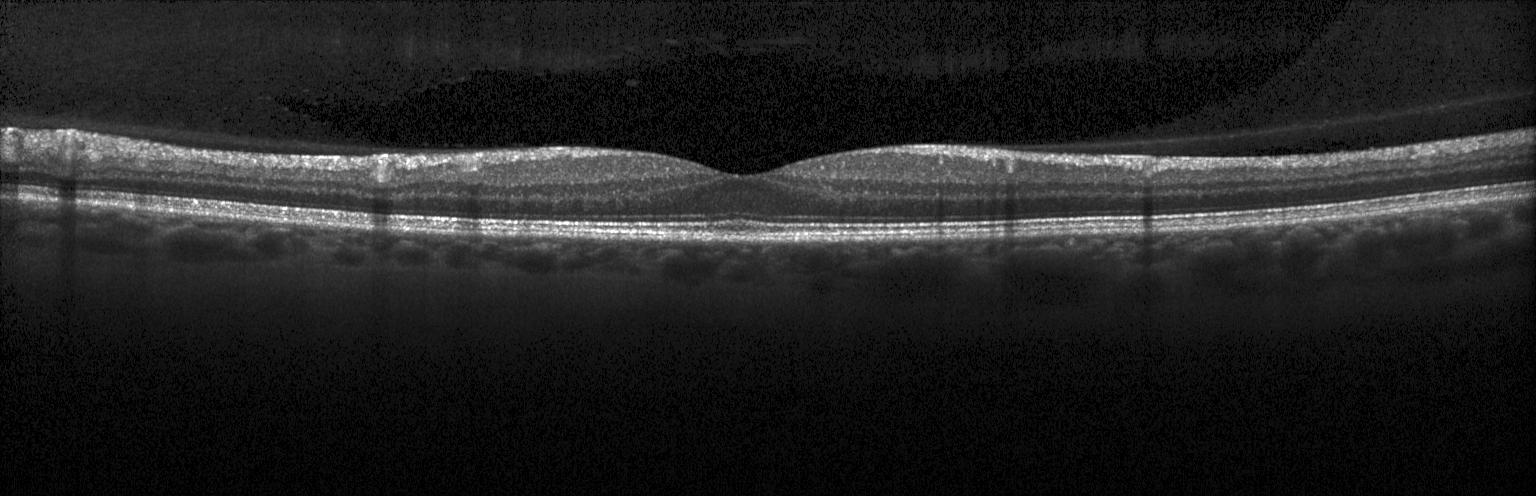
Macular OCT: no choroidal neovascularization, no diabetic macular edema, and no drusen.